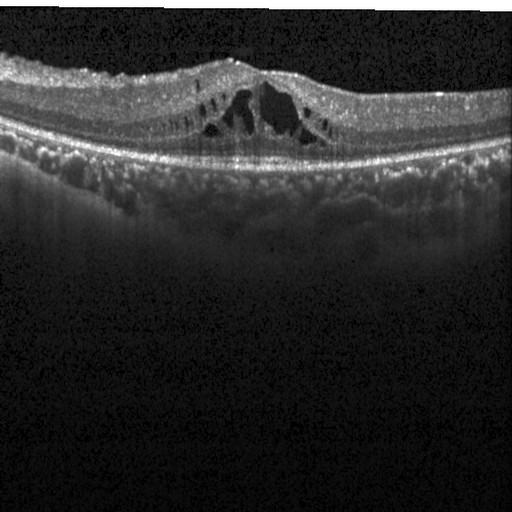 OCT finding: diabetic macular edema.